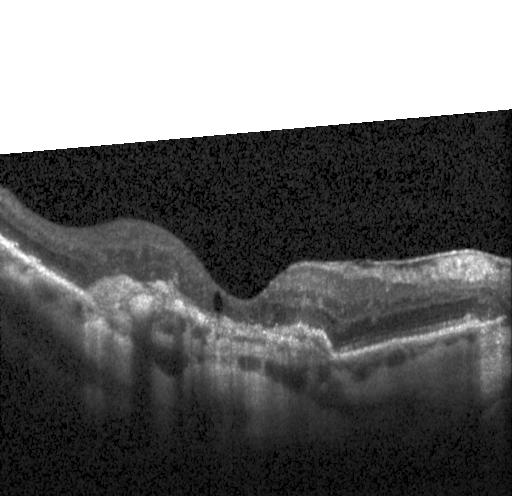

CNV.